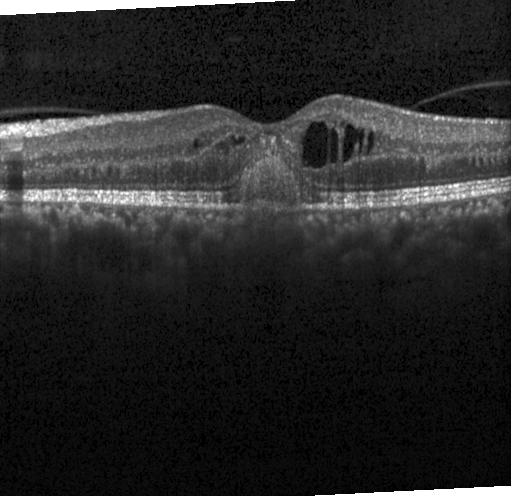

Macular scan · optical coherence tomography B-scan · acquired on a Heidelberg Spectralis — Assessment: a choroidal neovascular membrane.